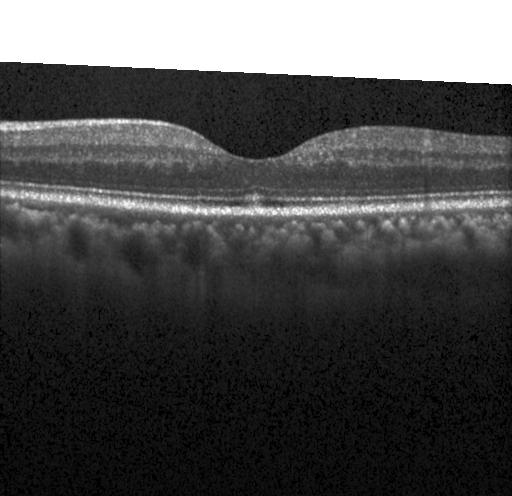 SD-OCT · centered on the fovea · retinal OCT cross-section · acquired on a Heidelberg Spectralis. OCT finding: neither choroidal neovascularization, diabetic macular edema, nor drusen.